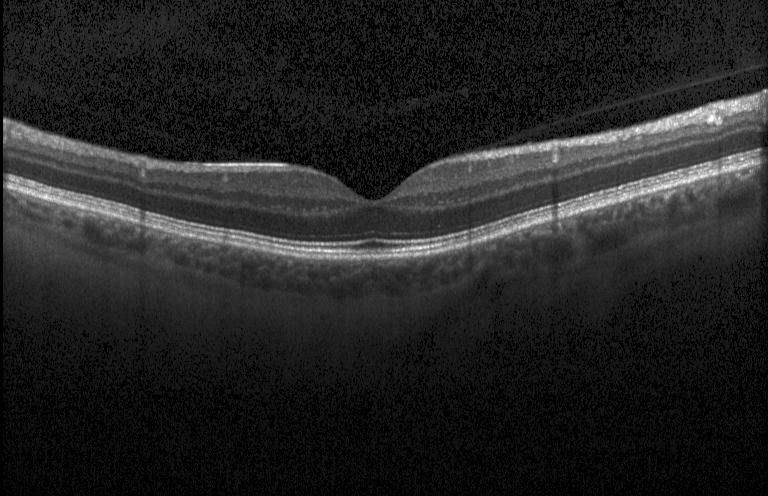
Heidelberg Spectralis · spectral-domain optical coherence tomography · OCT line scan · centered on the fovea
Impression: no evidence of choroidal neovascularization, diabetic macular edema, or drusen.